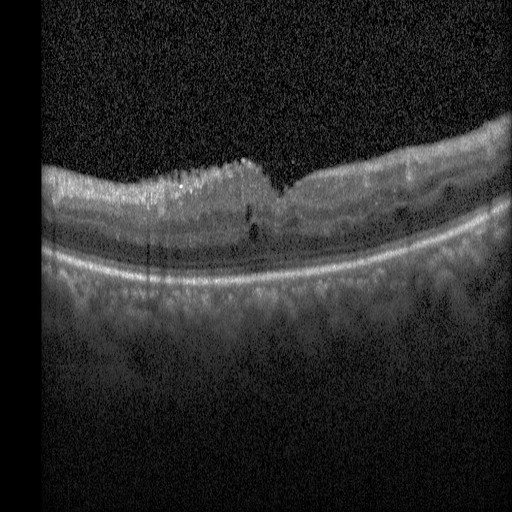 This B-scan demonstrates diabetic macular edema.